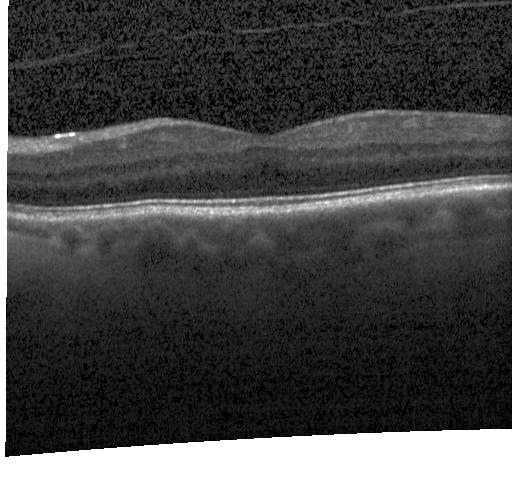
OCT finding: no choroidal neovascularization, no diabetic macular edema, and no drusen.